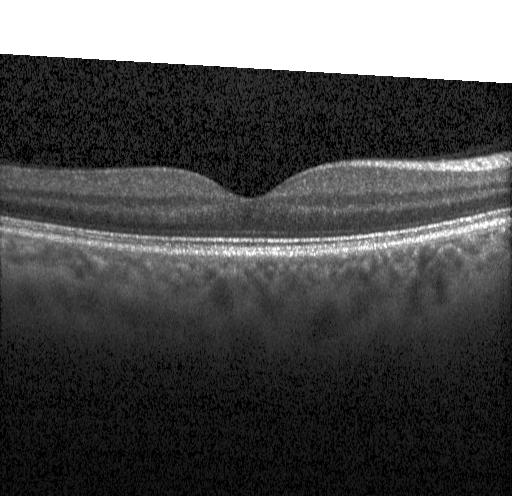 Horizontal scan through the fovea · OCT line scan
Diagnosis: no choroidal neovascularization, no diabetic macular edema, and no drusen.